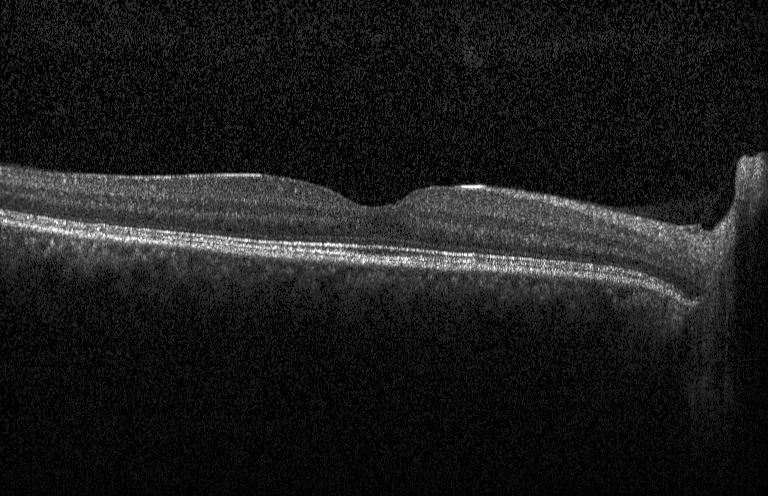
Assessment: no CNV, no DME, and no drusen.